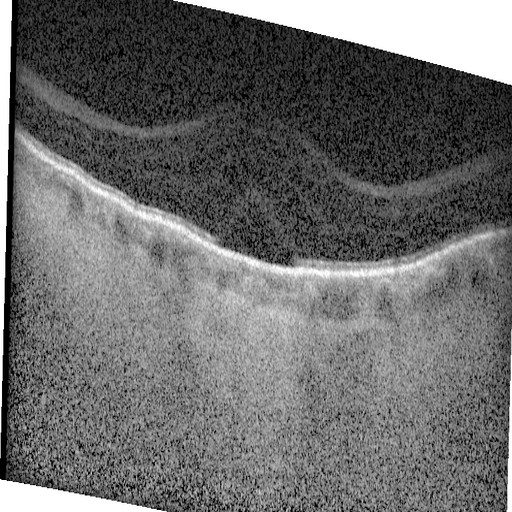 This B-scan demonstrates diabetic macular edema.